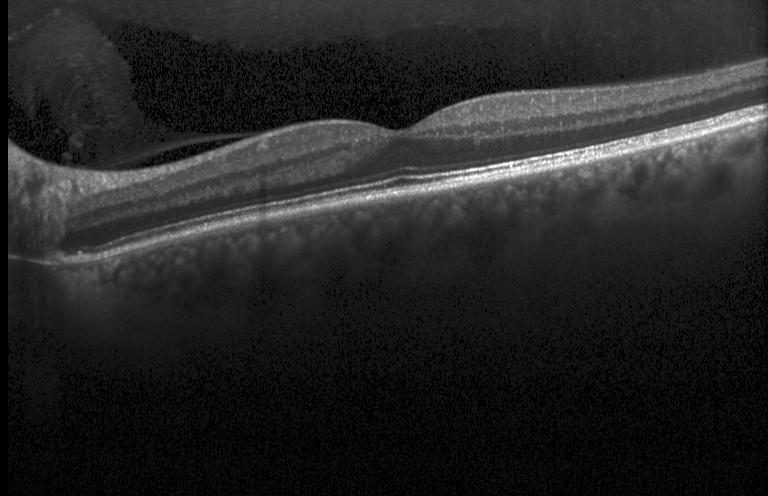
Finding: neither choroidal neovascularization, diabetic macular edema, nor drusen.